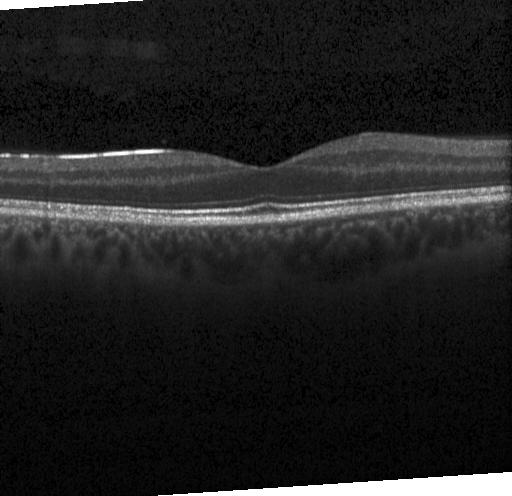 Retinal OCT cross-section, spectral-domain OCT
This B-scan demonstrates no evidence of CNV, DME, or drusen.